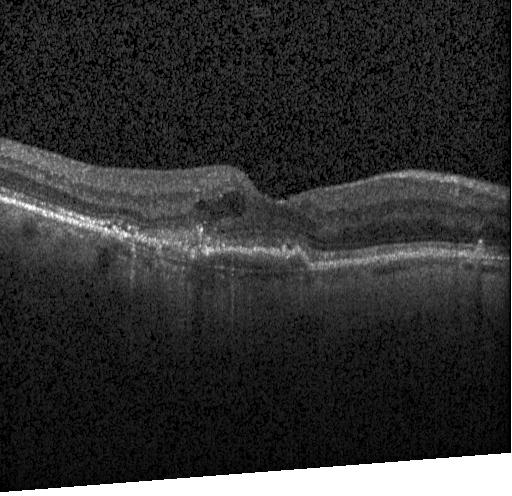 Dx: a choroidal neovascular membrane.